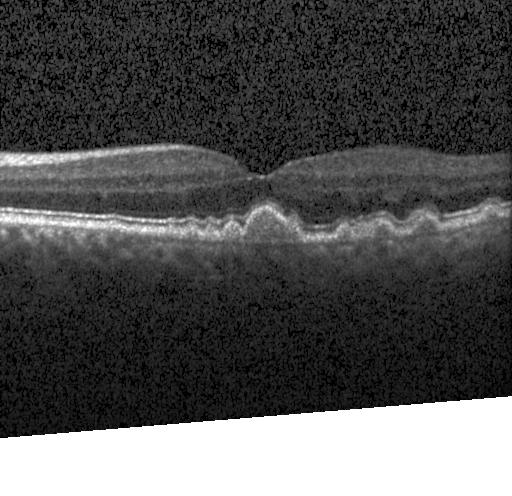

The scan shows multiple drusen.